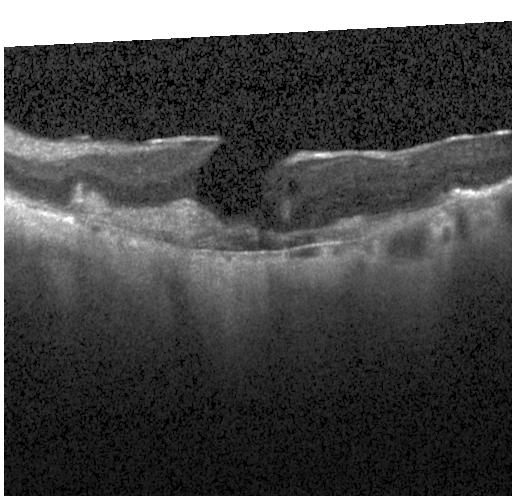

Acquired on a Heidelberg Spectralis, spectral-domain OCT, OCT line scan, centered on the fovea.
Assessment: a choroidal neovascular membrane.